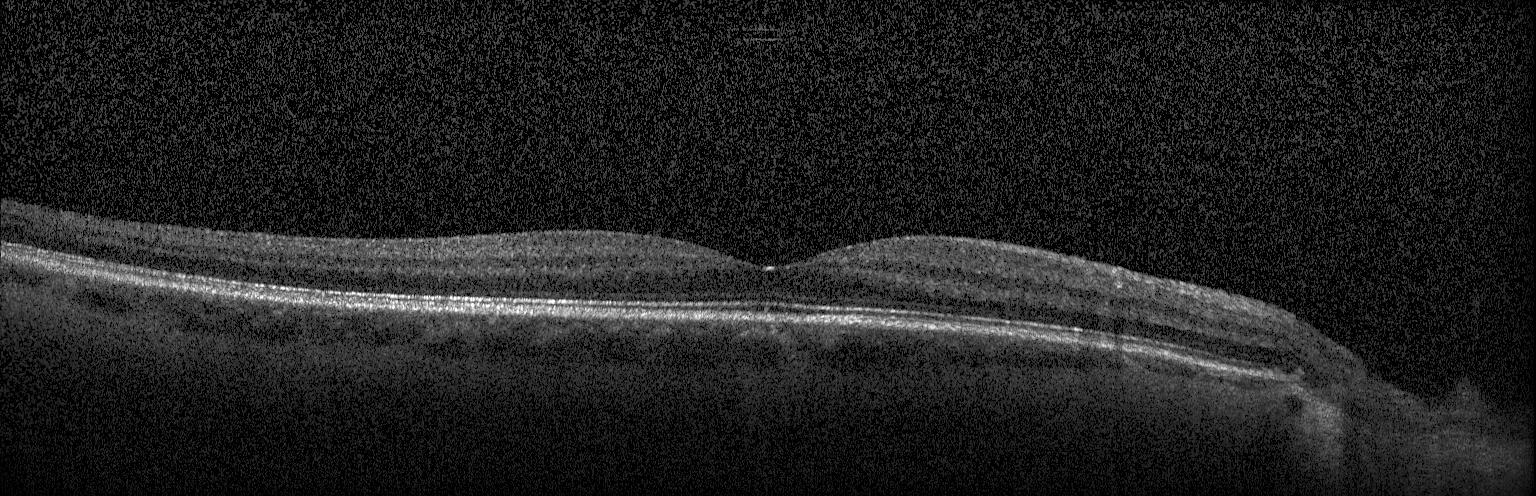

Instrument: Heidelberg Spectralis; spectral-domain optical coherence tomography; OCT line scan; horizontal scan through the fovea
Impression: no choroidal neovascularization, no diabetic macular edema, and no drusen.